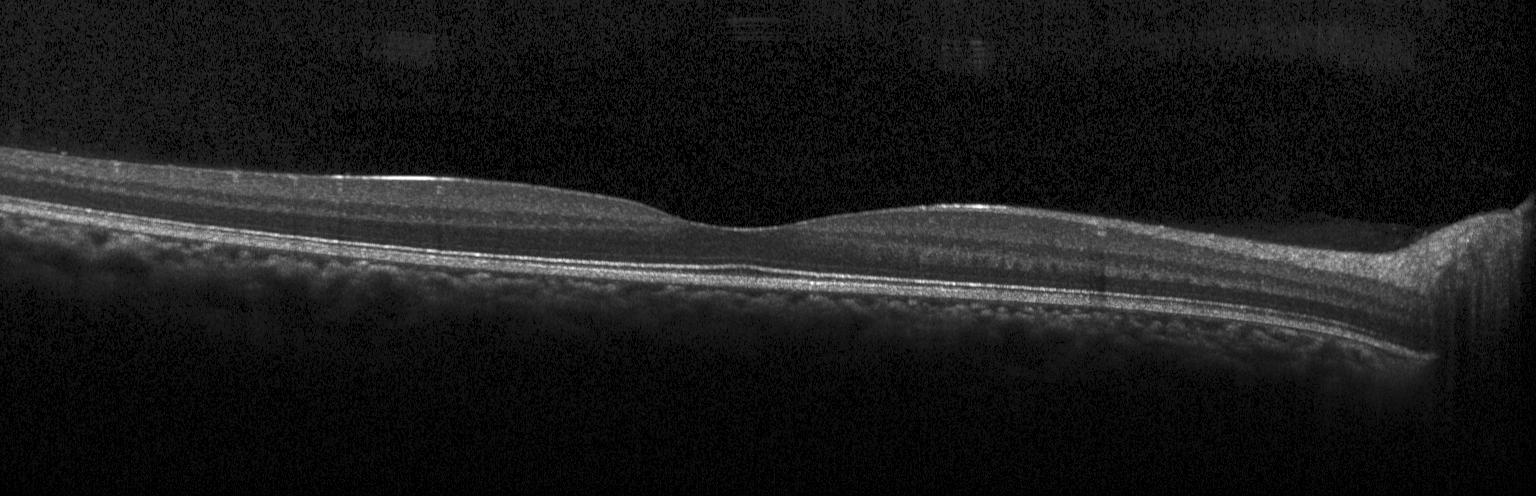

Fovea-centered; spectral-domain OCT; optical coherence tomography B-scan; instrument: Heidelberg Spectralis. Impression: no CNV, DME, or drusen.